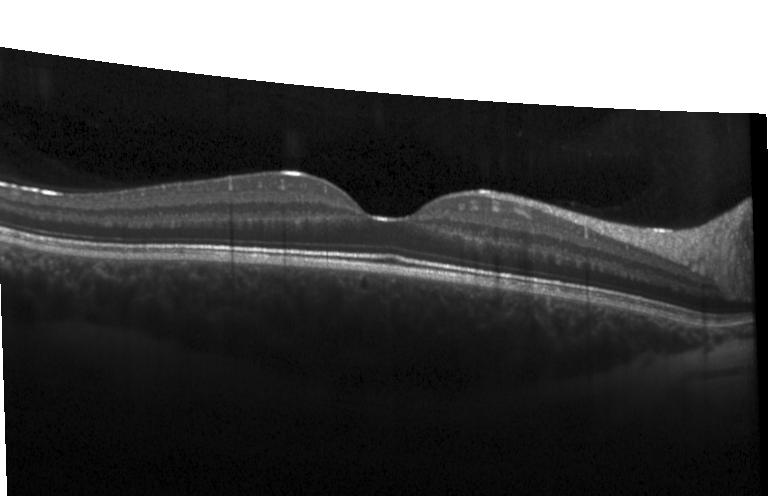
Optical coherence tomography B-scan, macular scan, Heidelberg Spectralis OCT system
Finding: no evidence of choroidal neovascularization, diabetic macular edema, or drusen.